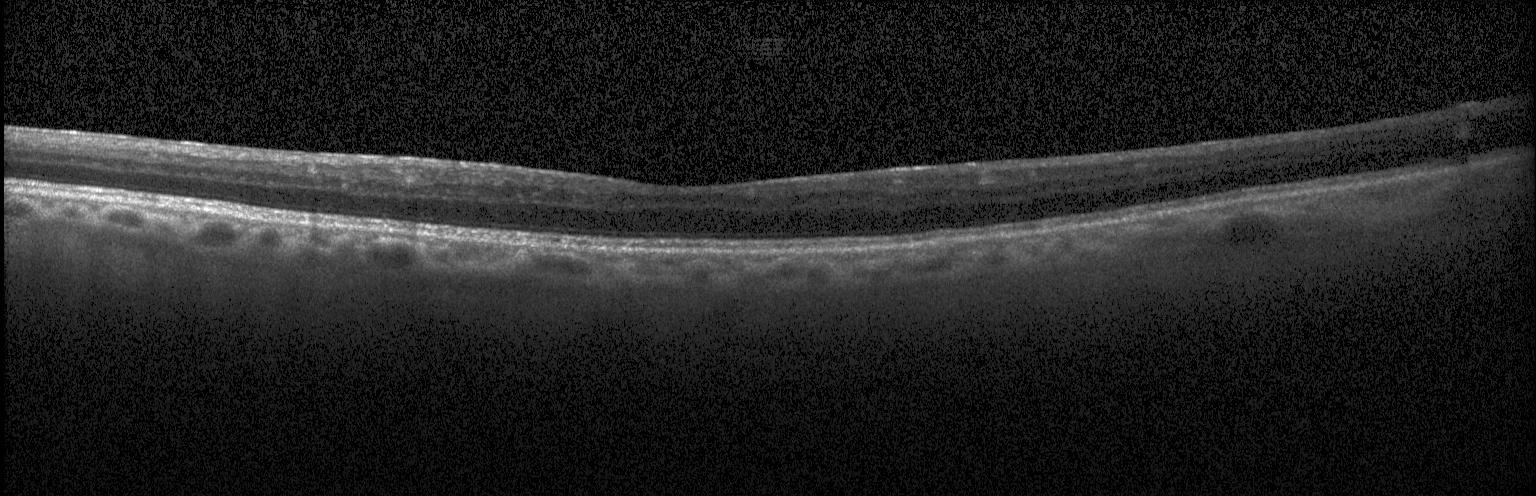 Spectral-domain optical coherence tomography, retinal OCT cross-section, through the macula.
Assessment: no evidence of choroidal neovascularization, diabetic macular edema, or drusen.